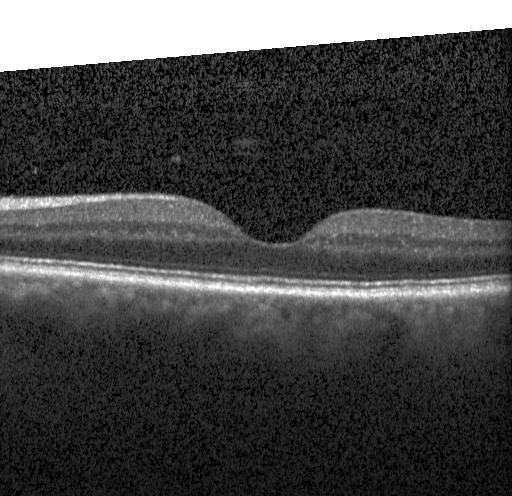

Dx: neither choroidal neovascularization, diabetic macular edema, nor drusen.